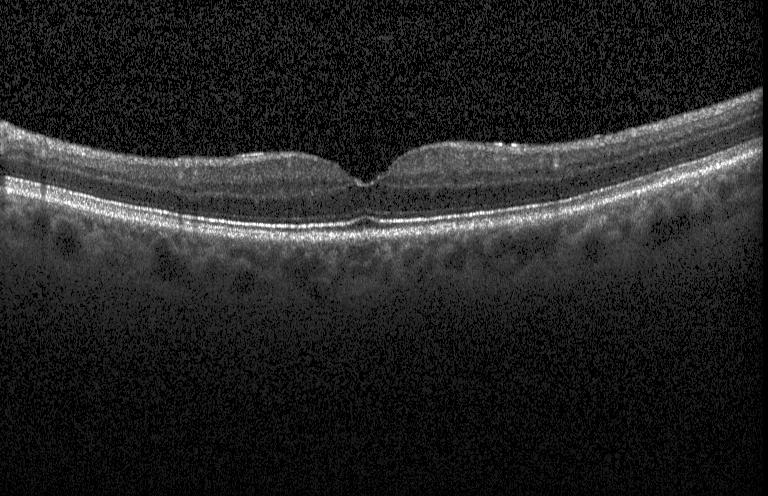 OCT scan showing neither CNV, DME, nor drusen.